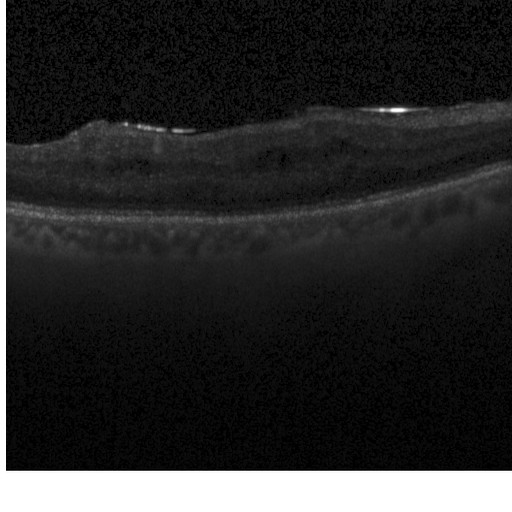 Impression: diabetic macular edema (DME).